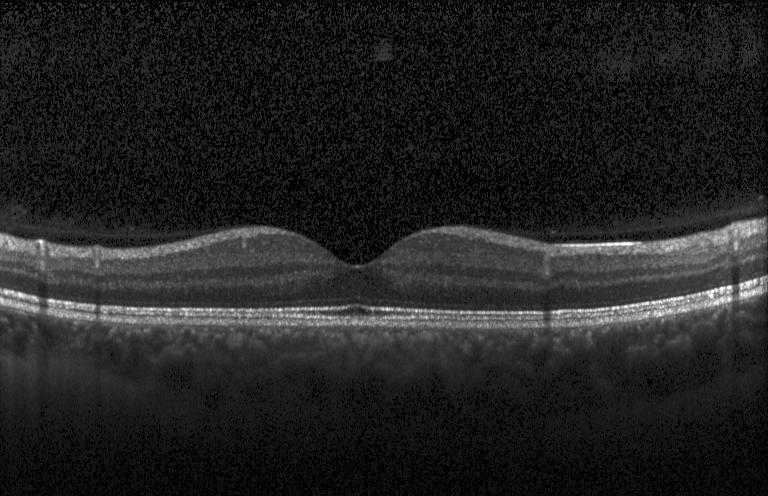 Diagnosis: no CNV, DME, or drusen.